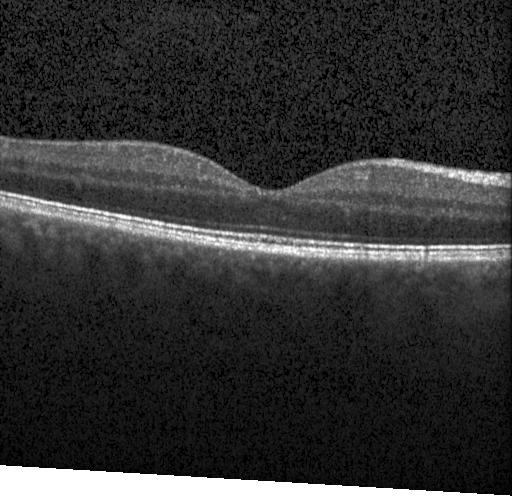 This B-scan demonstrates no CNV, no DME, and no drusen.